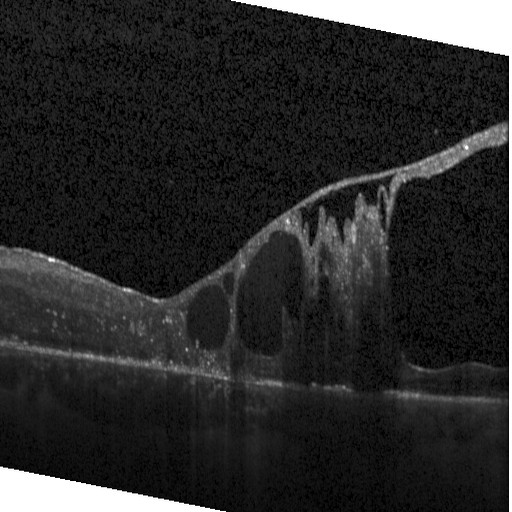 Optical coherence tomography scan.
Impression: DME.